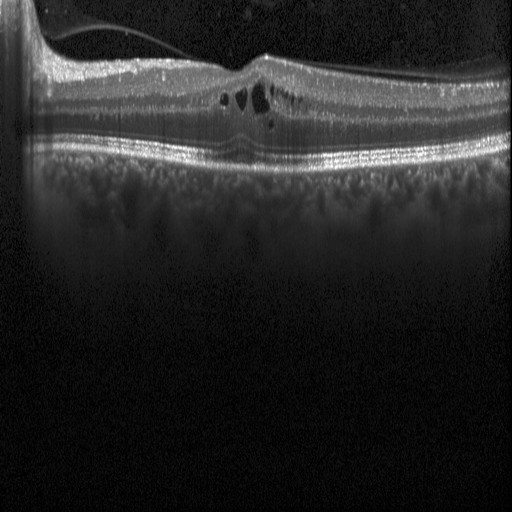
Spectral-domain OCT · retinal OCT cross-section · centered on the fovea · instrument: Heidelberg Spectralis.
OCT finding: diabetic macular edema (DME).